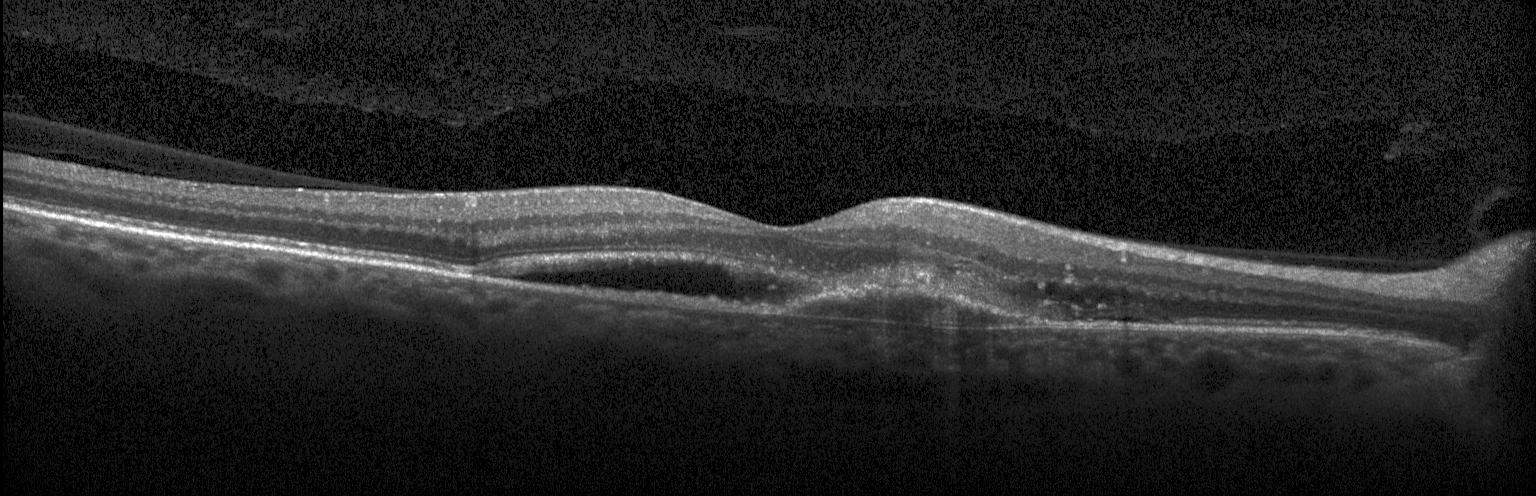 OCT scan showing choroidal neovascularization.